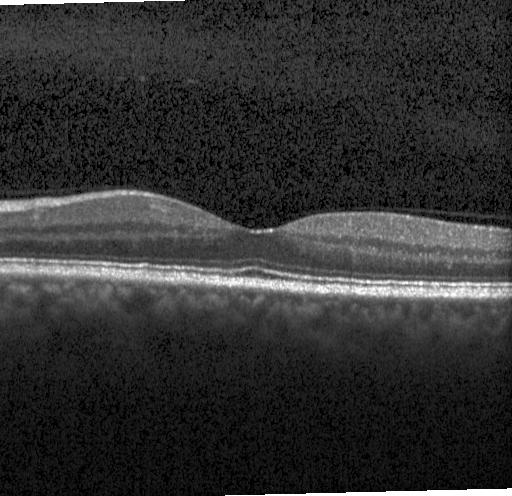

Diagnosis: no choroidal neovascularization, diabetic macular edema, or drusen.